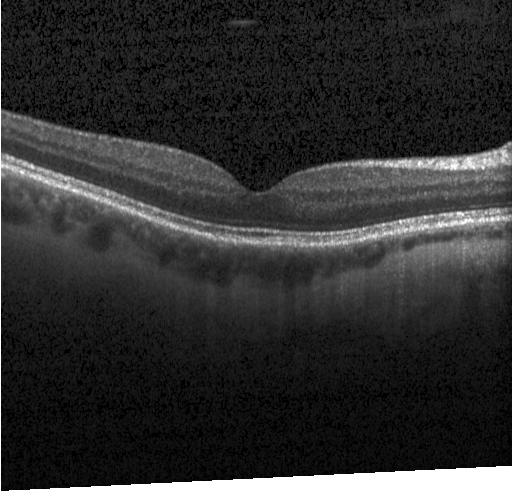

Assessment: no choroidal neovascularization, diabetic macular edema, or drusen.